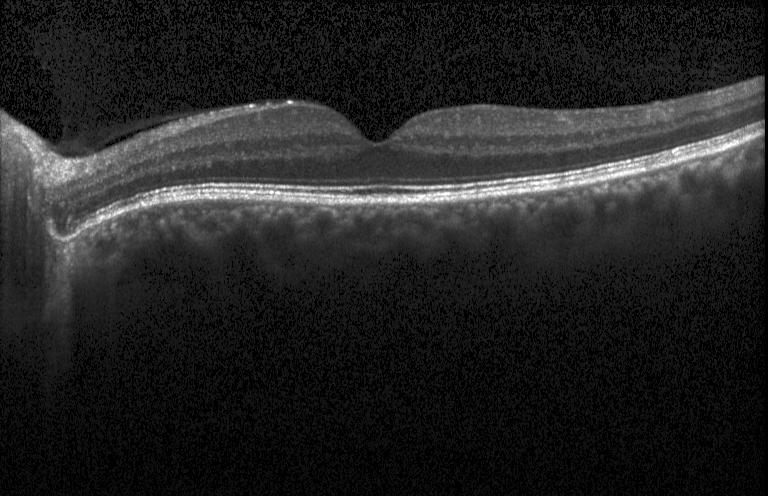
Finding: no CNV, no DME, and no drusen.